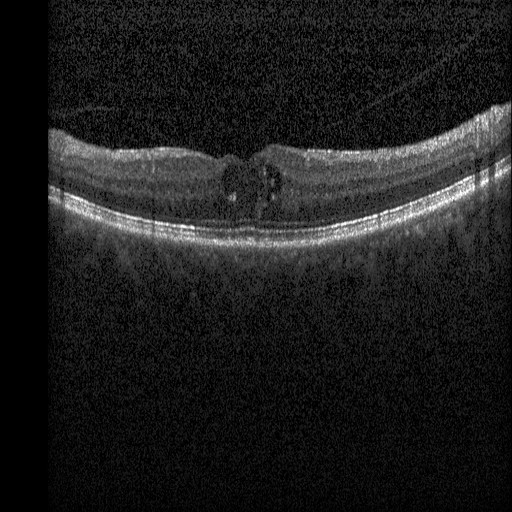

OCT finding: DME.